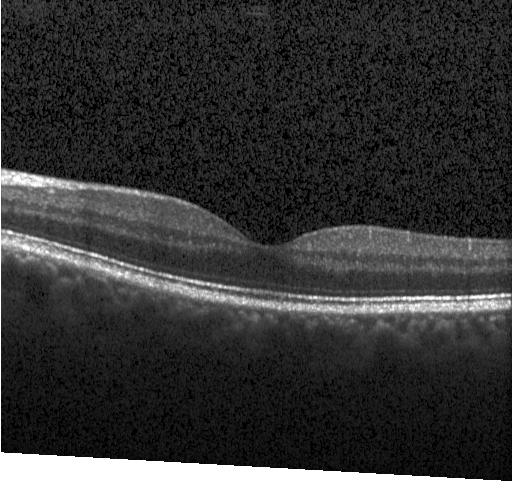 Dx: no evidence of CNV, DME, or drusen.